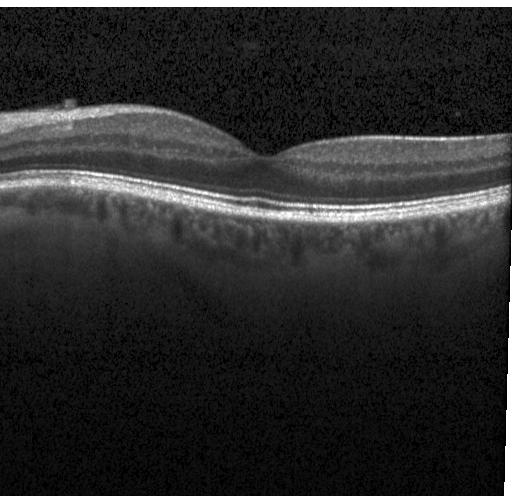
Retinal OCT B-scan, SD-OCT.
The scan shows neither choroidal neovascularization, diabetic macular edema, nor drusen.